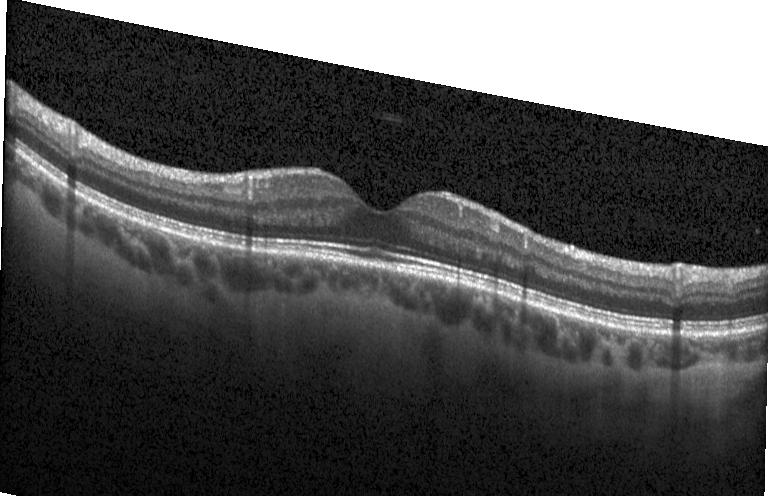

Diagnosis: no evidence of choroidal neovascularization, diabetic macular edema, or drusen.